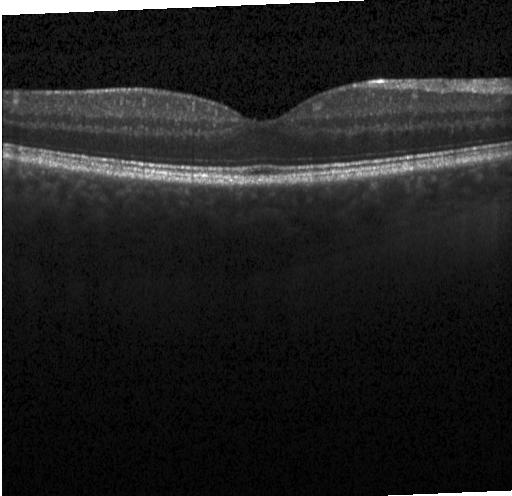
Macular OCT demonstrating no choroidal neovascularization, no diabetic macular edema, and no drusen.